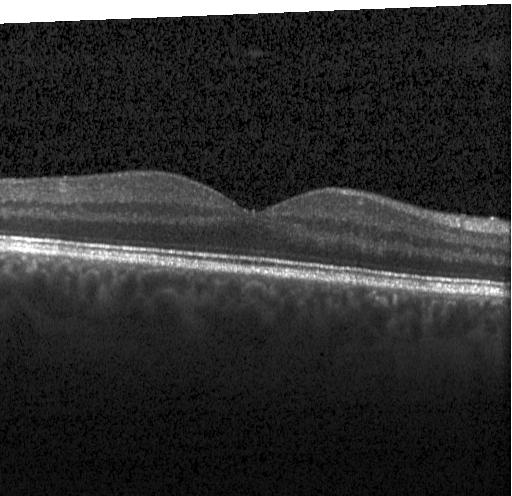
Retinal OCT cross-section showing no choroidal neovascularization, diabetic macular edema, or drusen.